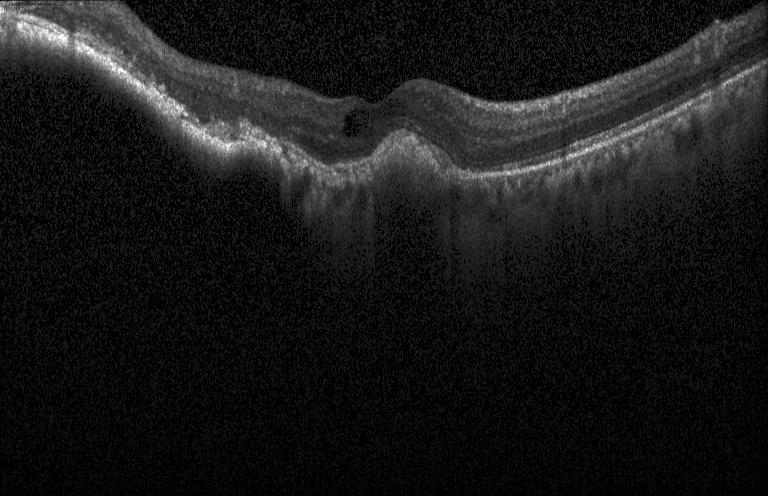
This B-scan demonstrates a choroidal neovascular membrane.